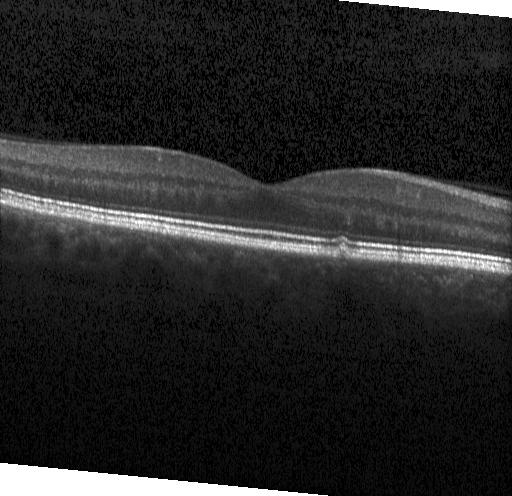 Impression: no evidence of choroidal neovascularization, diabetic macular edema, or drusen.